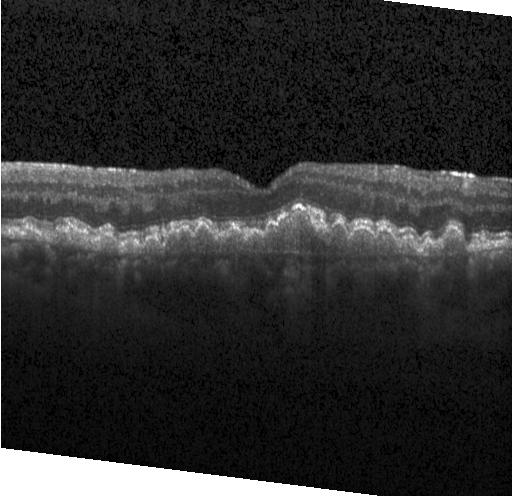 Diagnosis: CNV.